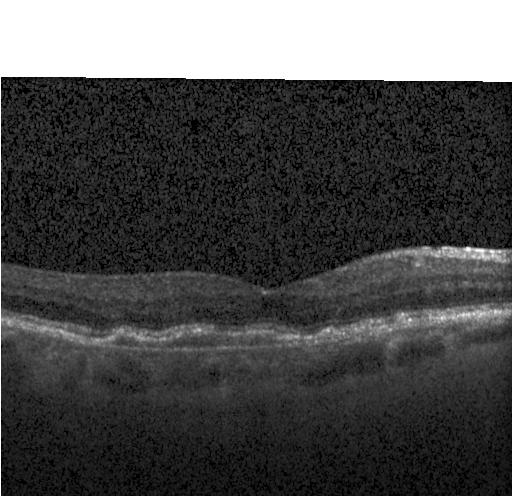
Finding: choroidal neovascularization.